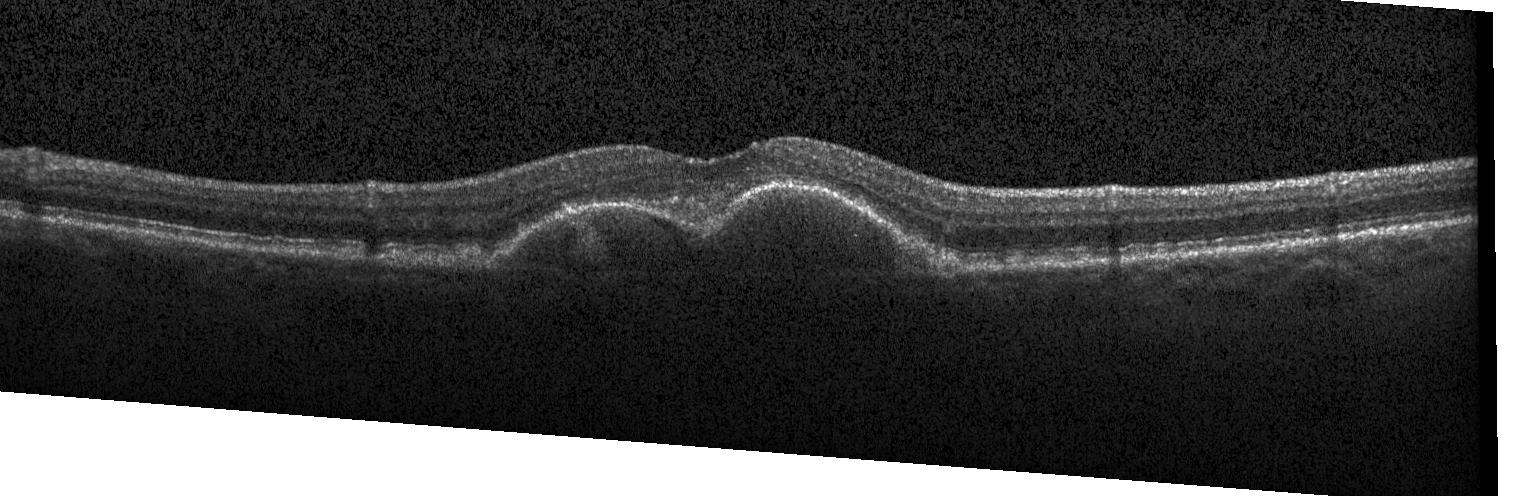 Heidelberg Spectralis · optical coherence tomography B-scan · SD-OCT · fovea-centered.
Impression: a choroidal neovascular membrane.